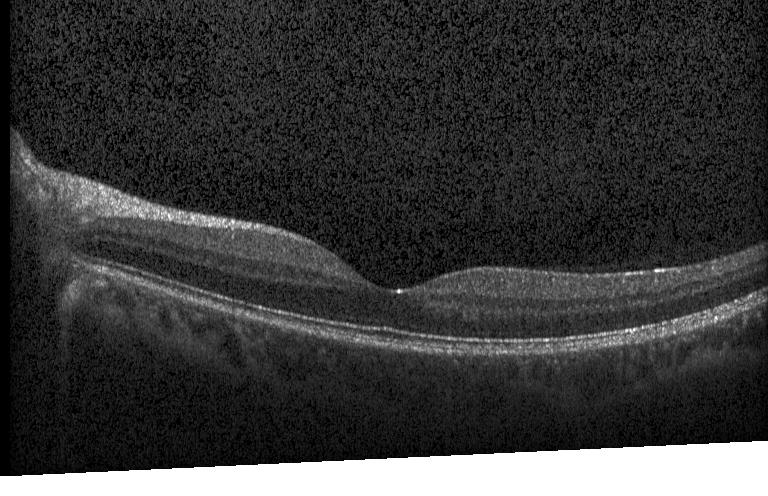
SD-OCT; retinal OCT cross-section; through the macula — Assessment: no evidence of choroidal neovascularization, diabetic macular edema, or drusen.